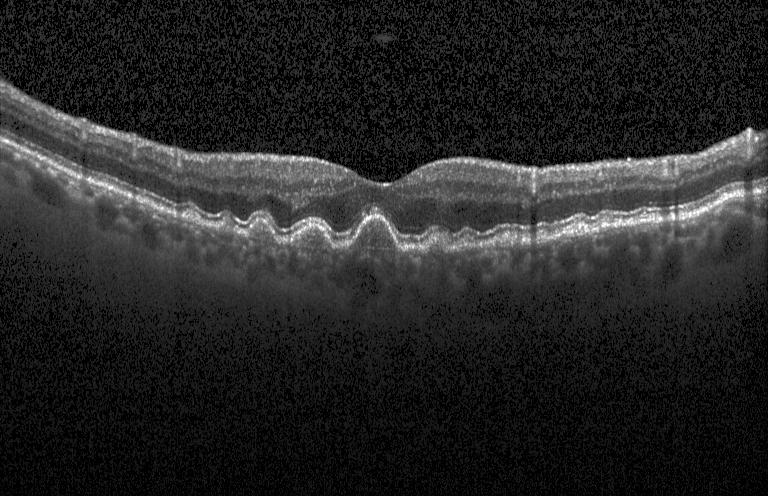 Optical coherence tomography B-scan. Multiple drusen.